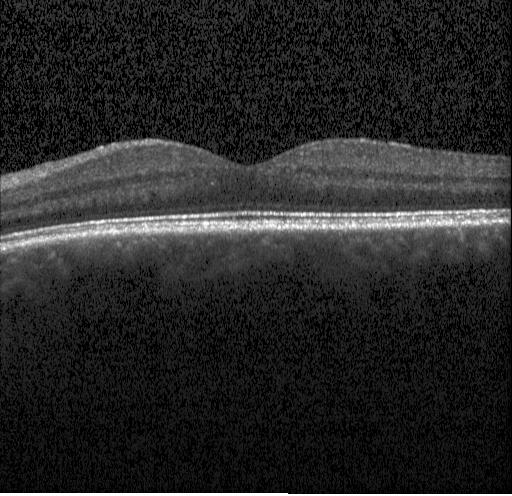

OCT B-scan · through the macula — This B-scan demonstrates no evidence of CNV, DME, or drusen.